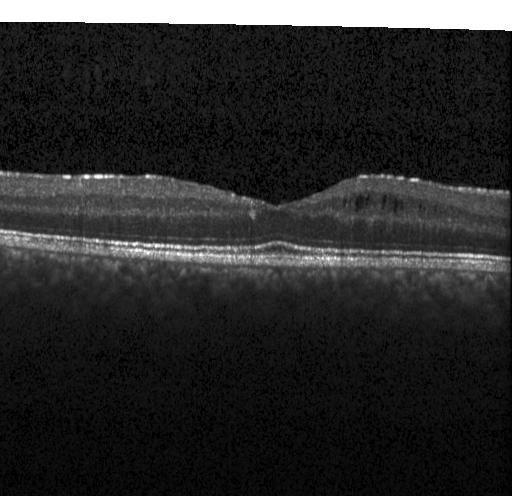

OCT line scan, SD-OCT, horizontal scan through the fovea, Heidelberg Spectralis. The scan shows diabetic macular edema (DME).